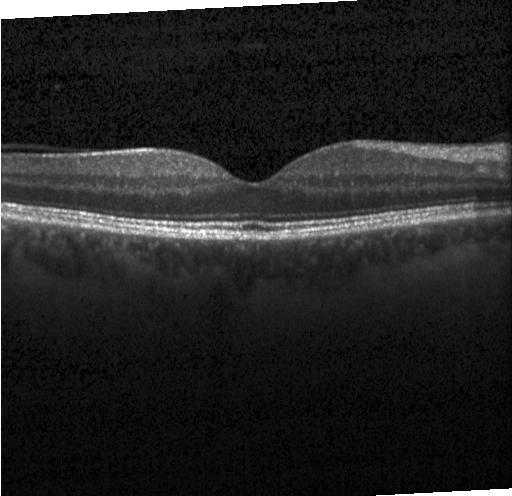
Finding: no evidence of CNV, DME, or drusen.